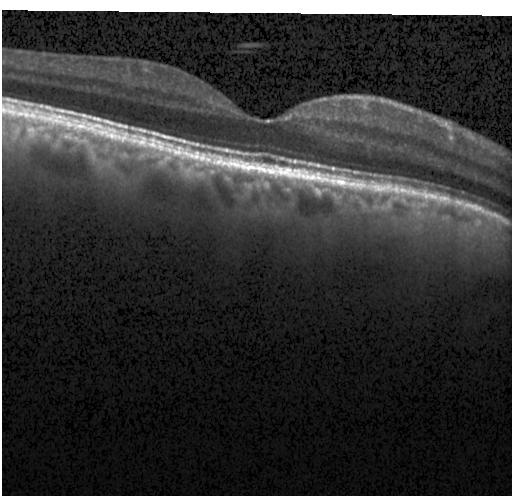 Horizontal scan through the fovea · OCT B-scan
Finding: no choroidal neovascularization, diabetic macular edema, or drusen.